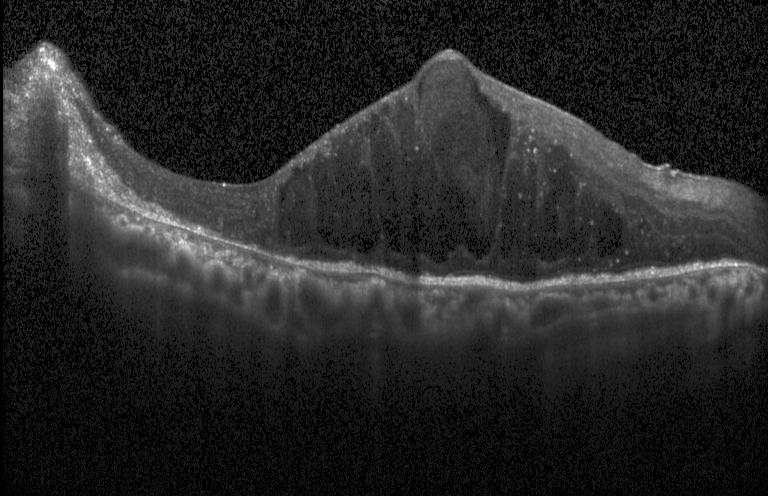

Retinal OCT cross-section. Instrument: Heidelberg Spectralis. Through the macula. This B-scan demonstrates DME.